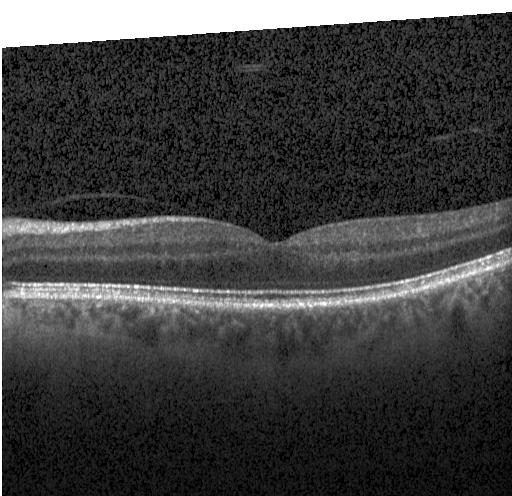 Macular OCT demonstrating neither choroidal neovascularization, diabetic macular edema, nor drusen.